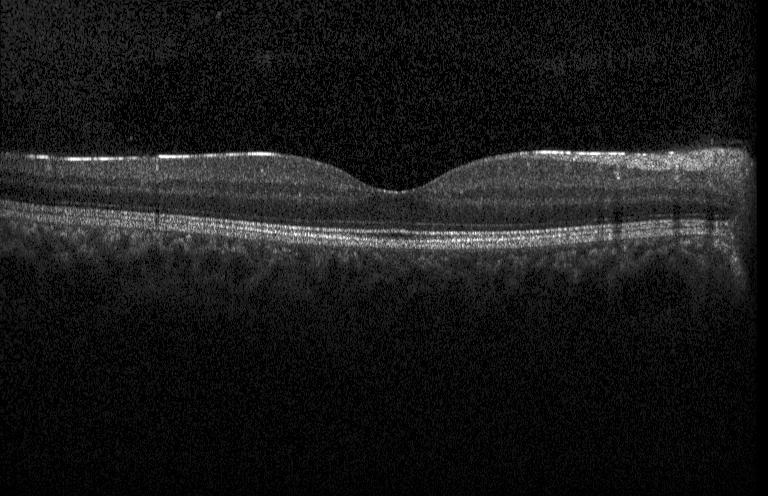

Optical coherence tomography scan. SD-OCT.
This B-scan demonstrates neither choroidal neovascularization, diabetic macular edema, nor drusen.